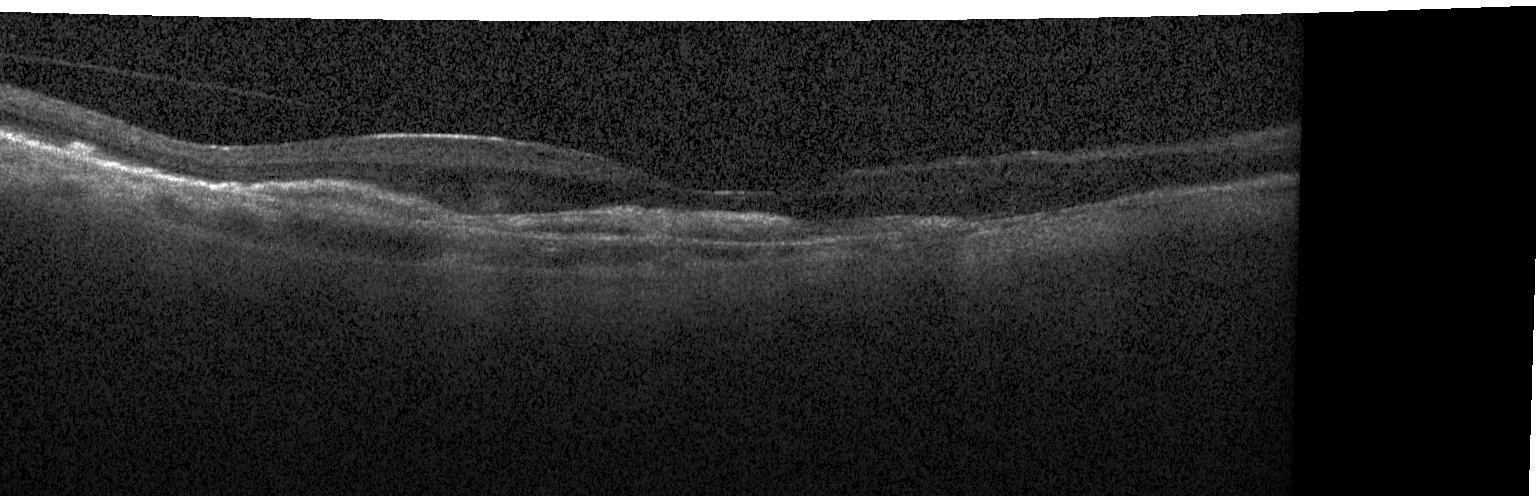 Optical coherence tomography B-scan.
Diagnosis: choroidal neovascularization (CNV).